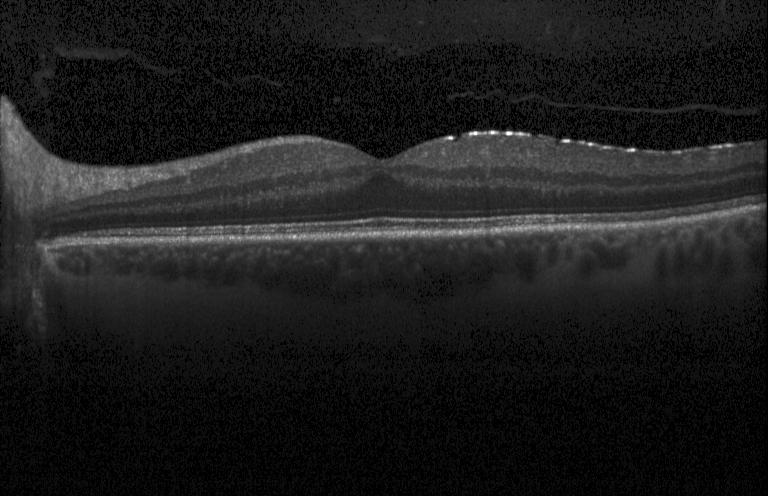
Acquired on a Heidelberg Spectralis. Centered on the fovea. SD-OCT. Retinal OCT B-scan
Diagnosis: no CNV, no DME, and no drusen.